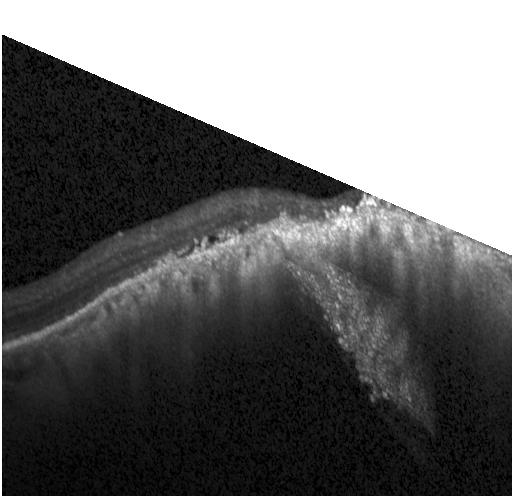 Macular OCT: a choroidal neovascular membrane.